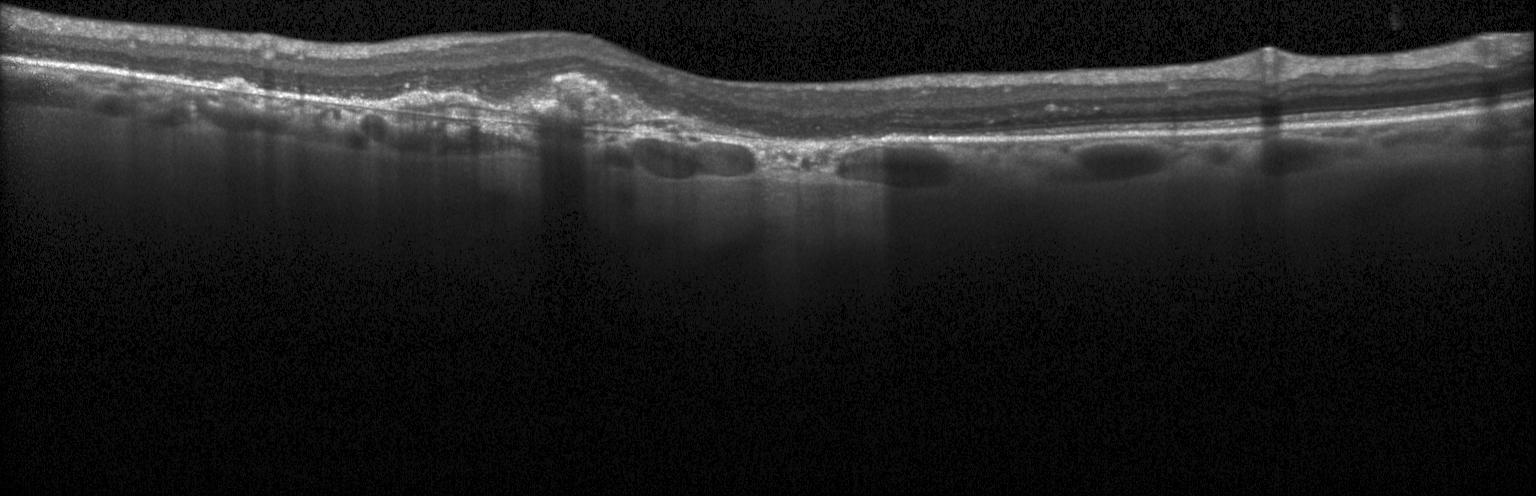
OCT B-scan — This B-scan demonstrates a choroidal neovascular membrane.